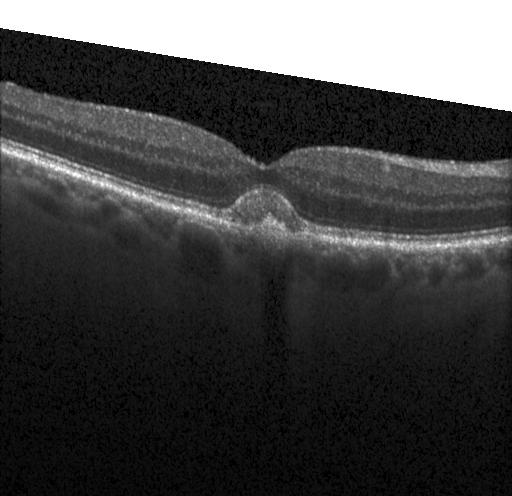 Diagnosis: CNV.